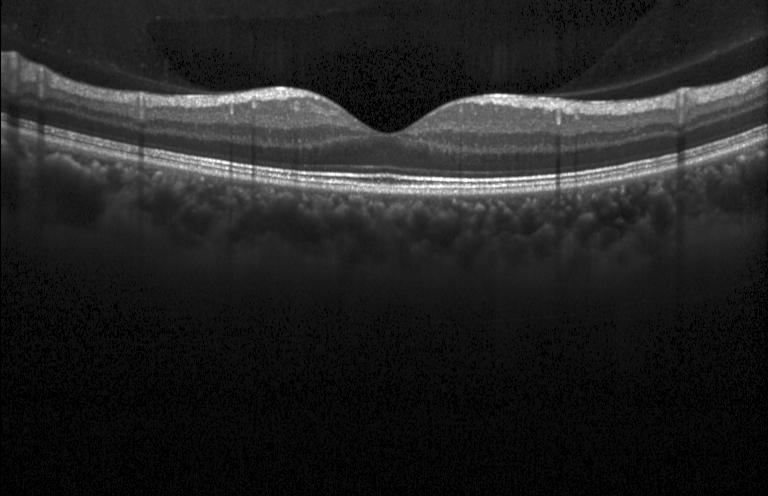 Retinal OCT cross-section.
Diagnosis: neither choroidal neovascularization, diabetic macular edema, nor drusen.